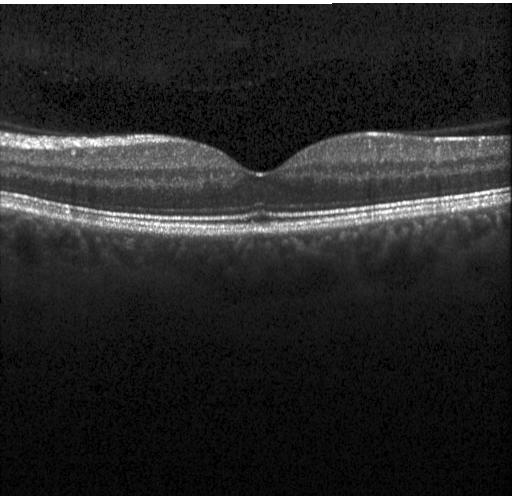
Heidelberg Spectralis OCT system, centered on the fovea, retinal OCT cross-section, spectral-domain OCT
Finding: no choroidal neovascularization, no diabetic macular edema, and no drusen.